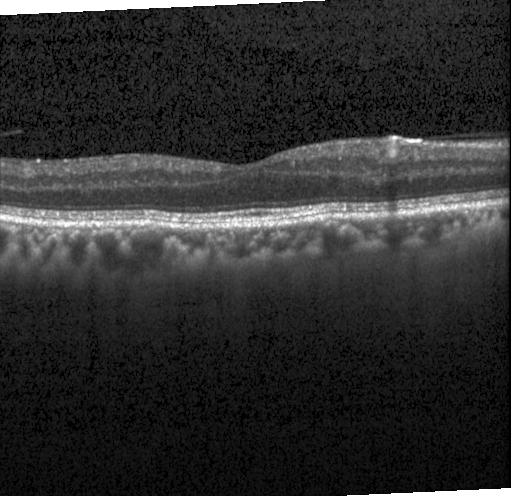 OCT line scan, Heidelberg Spectralis OCT system.
Macular OCT: neither choroidal neovascularization, diabetic macular edema, nor drusen.